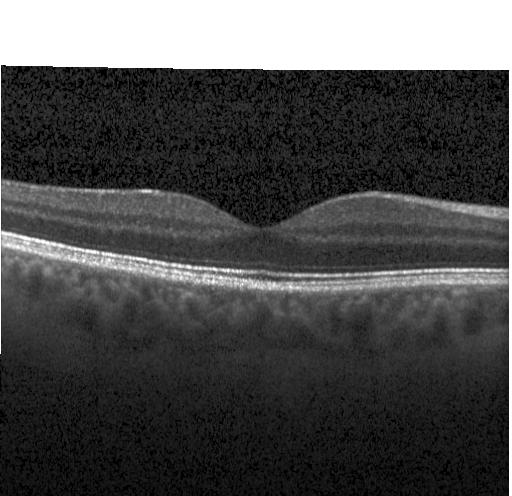 Dx: no CNV, no DME, and no drusen.